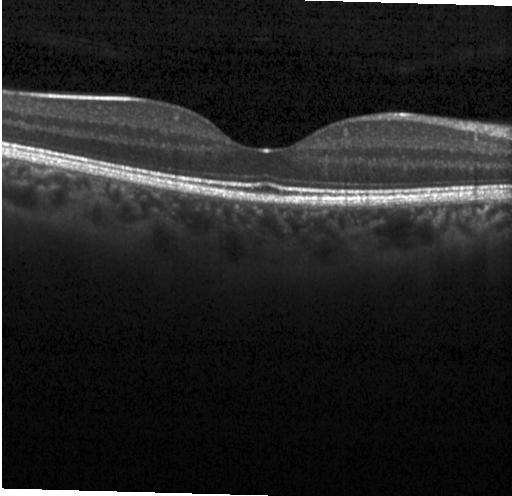

Spectral-domain OCT; instrument: Heidelberg Spectralis; centered on the fovea; OCT B-scan
Impression: no choroidal neovascularization, no diabetic macular edema, and no drusen.